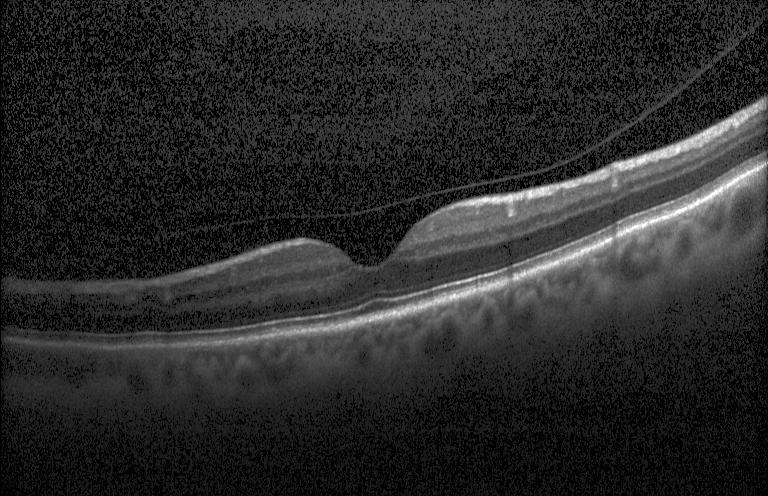
OCT line scan — Impression: no evidence of choroidal neovascularization, diabetic macular edema, or drusen.